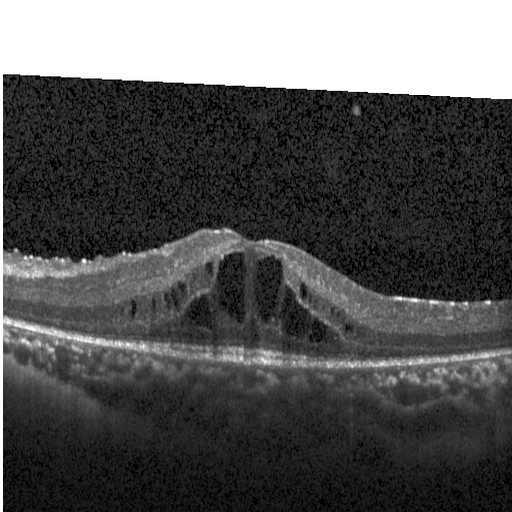

Macular OCT: DME.